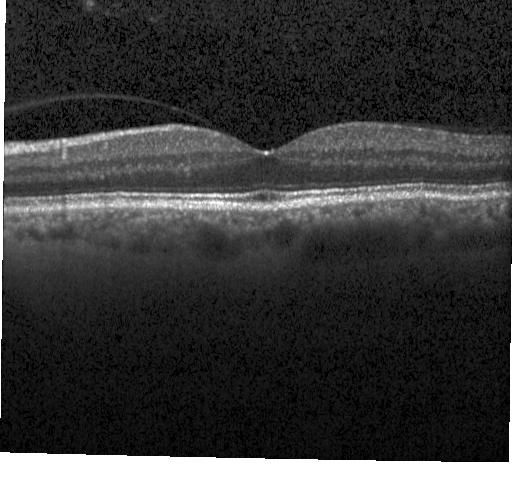

Macular OCT: no evidence of CNV, DME, or drusen.